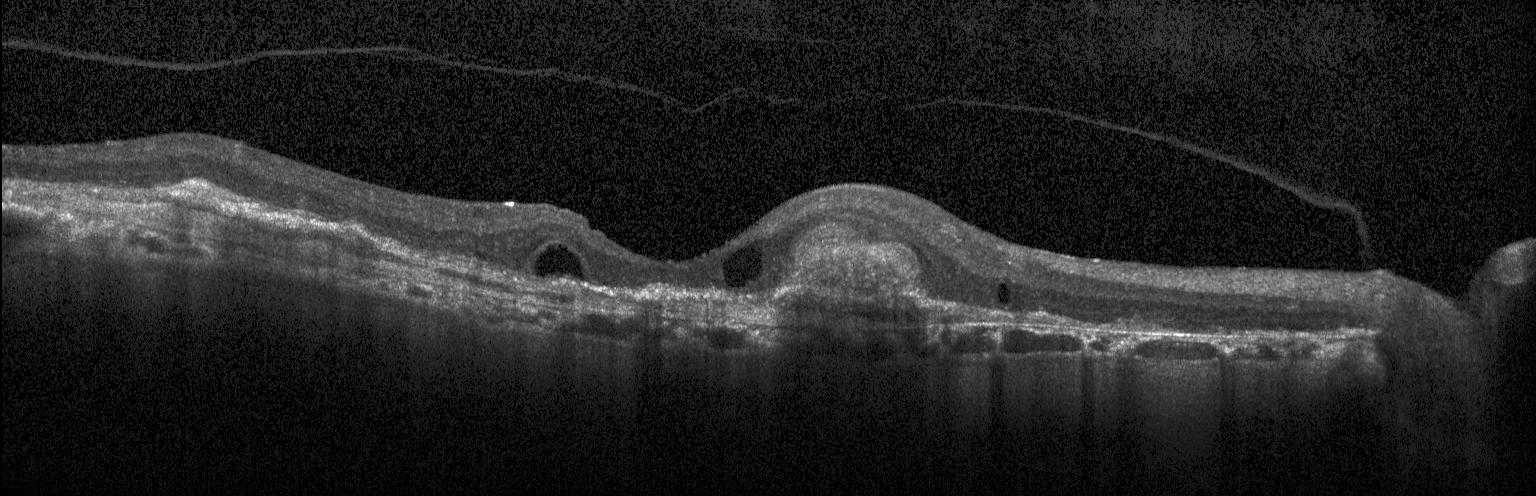

Retinal OCT B-scan — Finding: a choroidal neovascular membrane.